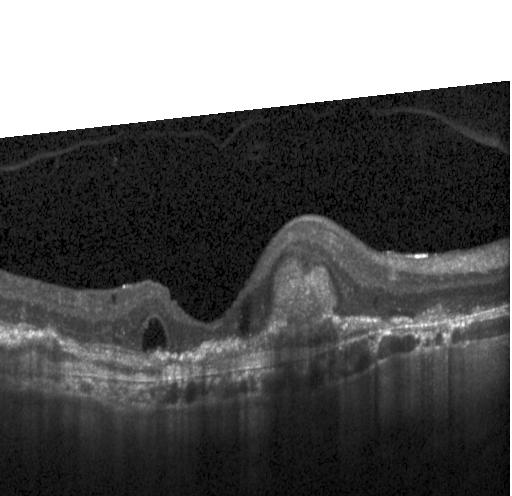

The scan shows a choroidal neovascular membrane.